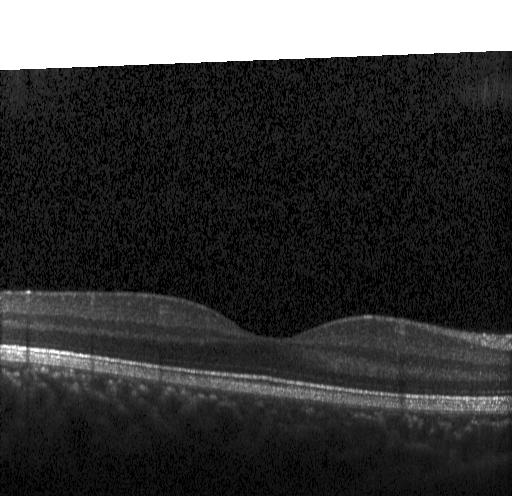
Retinal OCT cross-section · SD-OCT · Heidelberg Spectralis · horizontal scan through the fovea. No evidence of choroidal neovascularization, diabetic macular edema, or drusen.